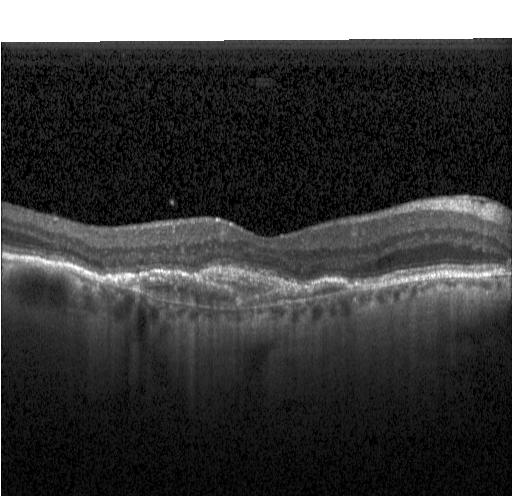

Retinal OCT cross-section · macular scan
This B-scan demonstrates a choroidal neovascular membrane.